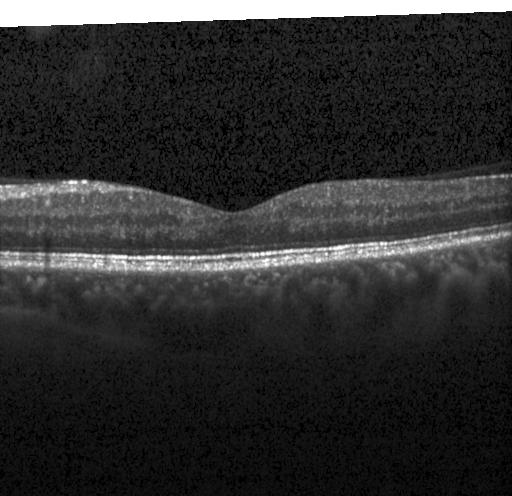

Retinal OCT cross-section showing no evidence of CNV, DME, or drusen.